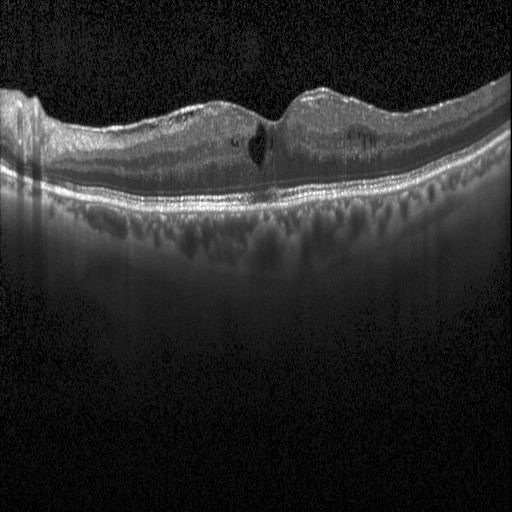

Impression: diabetic macular edema.